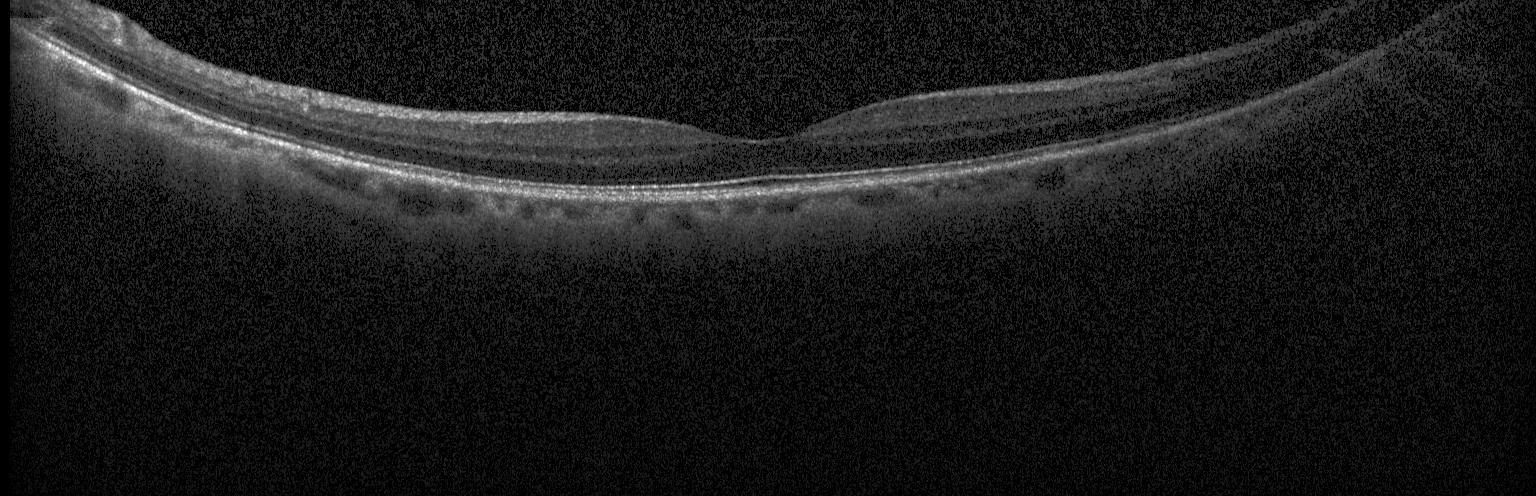 Spectral-domain optical coherence tomography. Through the macula. Retinal OCT cross-section.
This B-scan demonstrates no choroidal neovascularization, diabetic macular edema, or drusen.